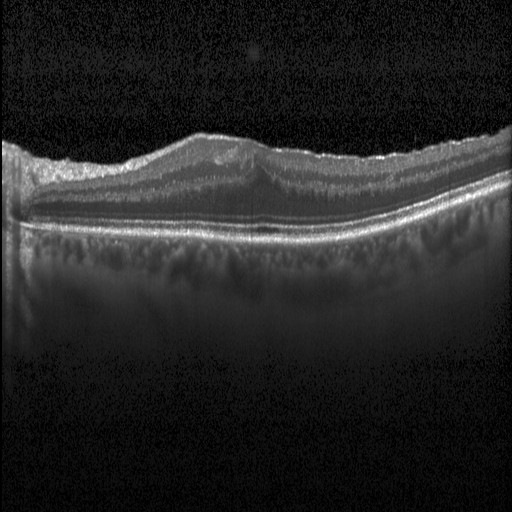
Retinal OCT cross-section. Macular scan. SD-OCT. Heidelberg Spectralis OCT system — DME.